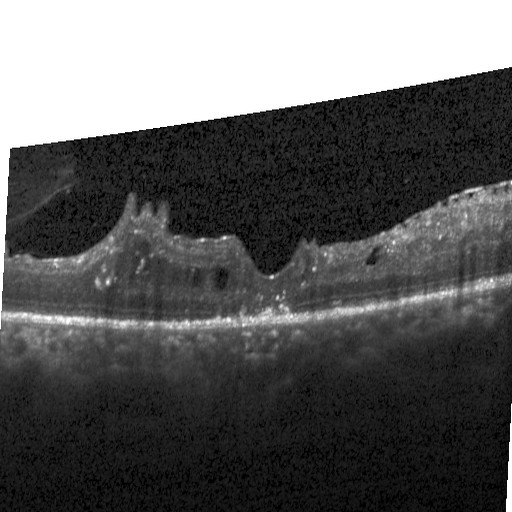 Optical coherence tomography B-scan · instrument: Heidelberg Spectralis — The scan shows diabetic macular edema.